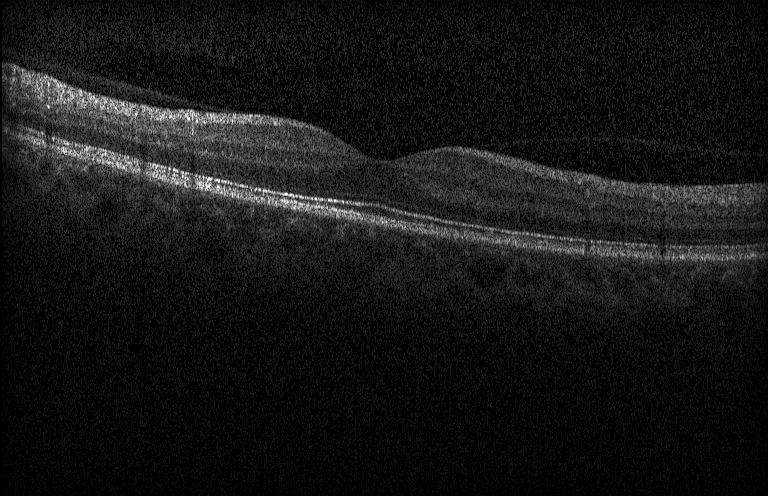 Diagnosis: no evidence of choroidal neovascularization, diabetic macular edema, or drusen.